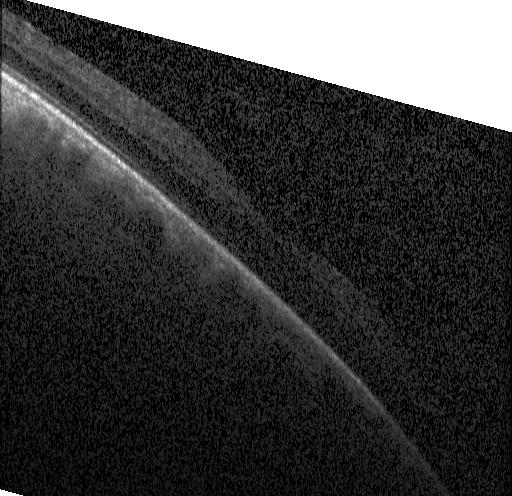
Macular OCT: neither CNV, DME, nor drusen.